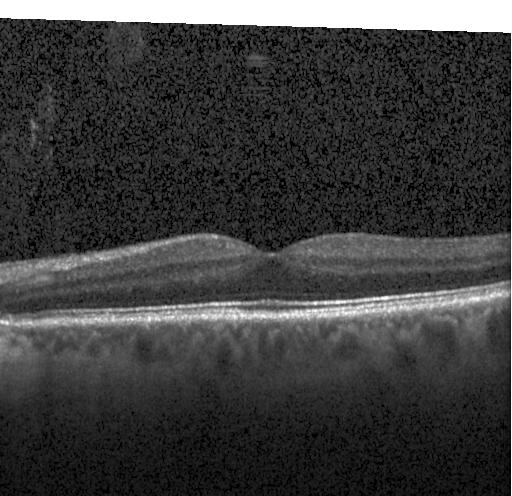 Retinal OCT B-scan · spectral-domain optical coherence tomography — Finding: no choroidal neovascularization, diabetic macular edema, or drusen.